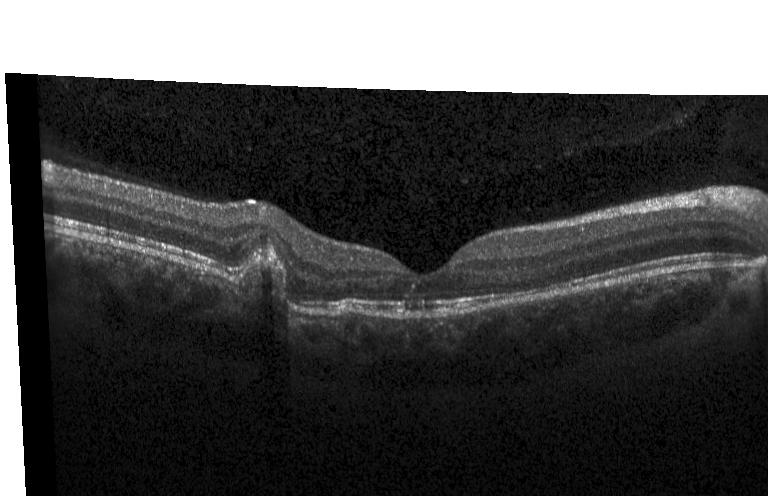
Optical coherence tomography scan, instrument: Heidelberg Spectralis — OCT finding: choroidal neovascularization (CNV).